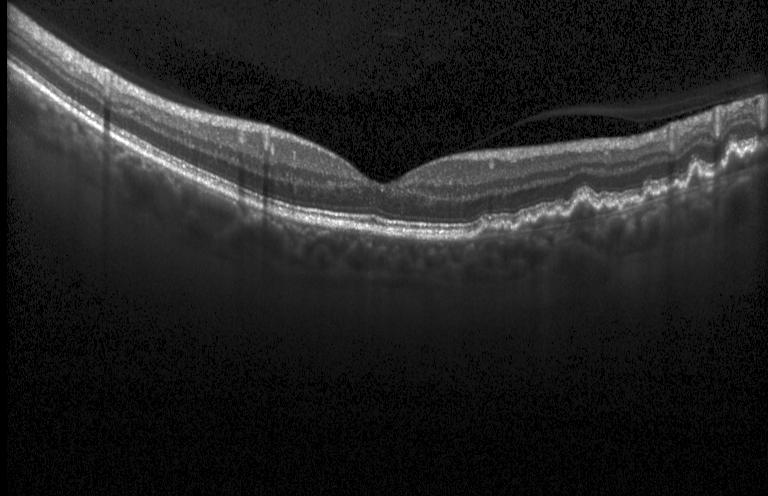 OCT B-scan showing a choroidal neovascular membrane.